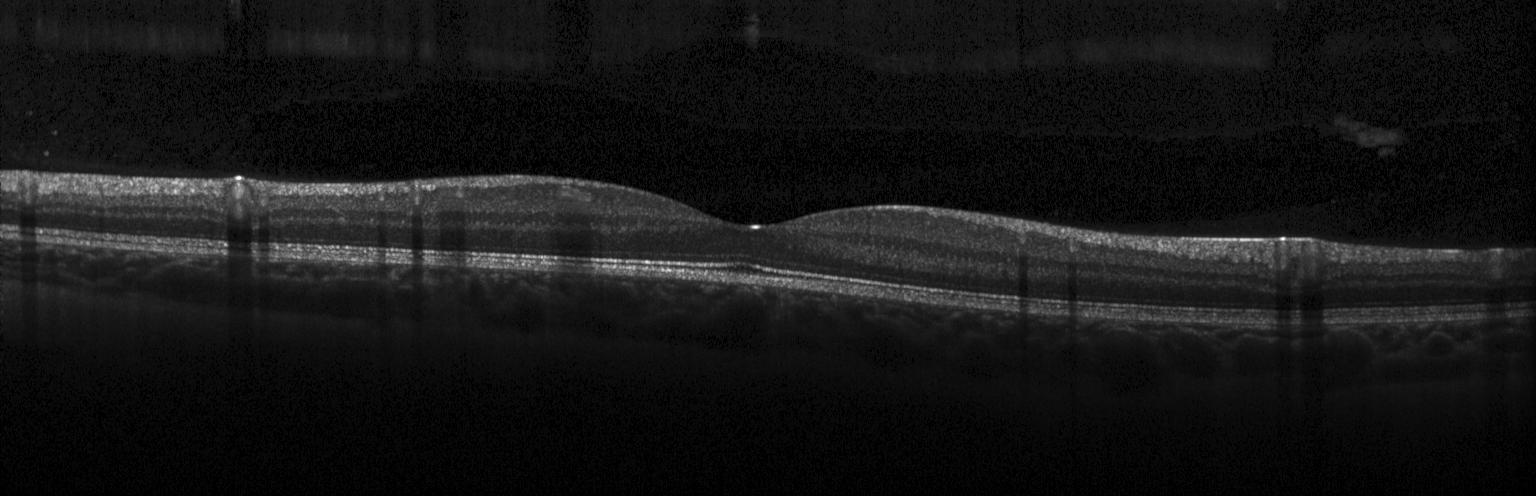 OCT B-scan
The scan shows neither choroidal neovascularization, diabetic macular edema, nor drusen.